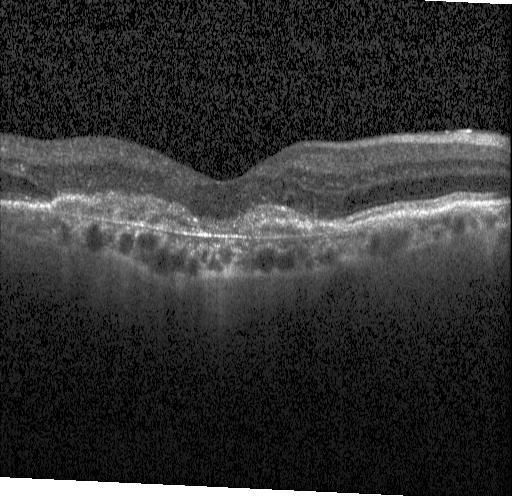 Retinal OCT cross-section · acquired on a Heidelberg Spectralis · through the macula.
The scan shows a choroidal neovascular membrane.